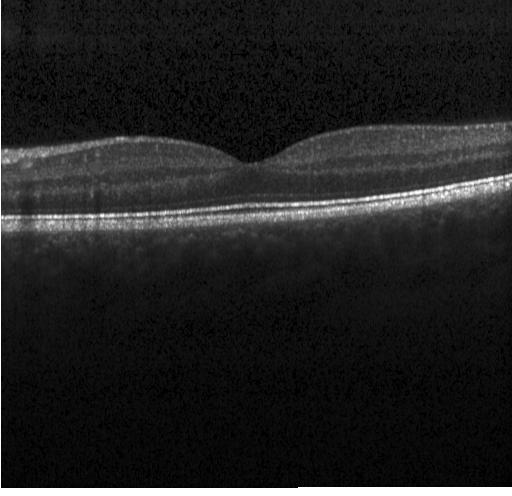
Horizontal scan through the fovea · OCT B-scan · spectral-domain OCT · instrument: Heidelberg Spectralis — Finding: no evidence of choroidal neovascularization, diabetic macular edema, or drusen.